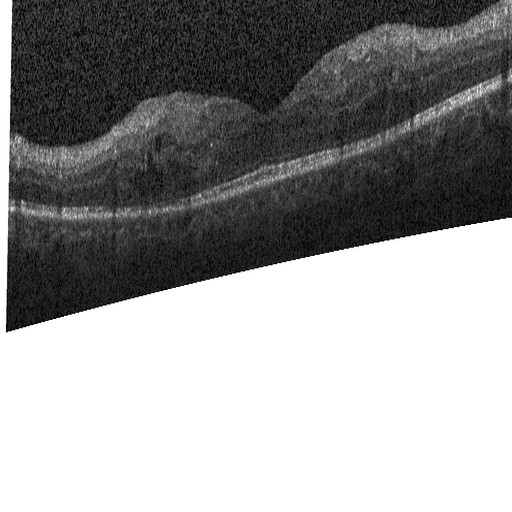

OCT B-scan; SD-OCT; horizontal scan through the fovea. Diagnosis: diabetic macular edema (DME).